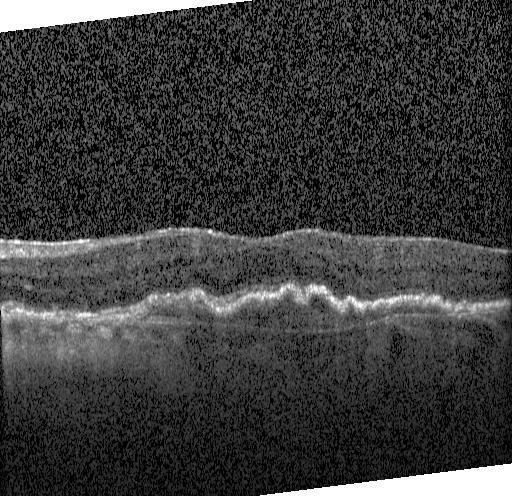 OCT scan showing choroidal neovascularization.